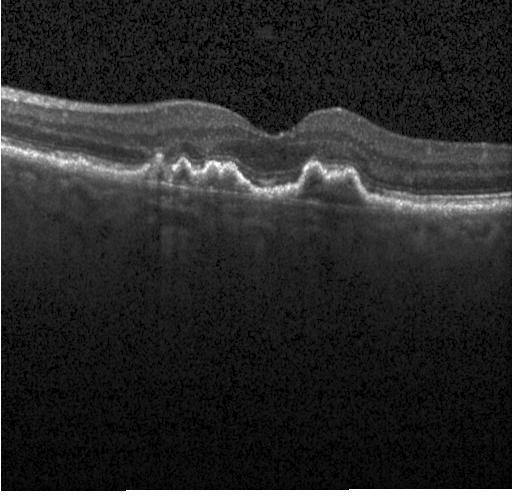

Retinal OCT cross-section showing CNV.